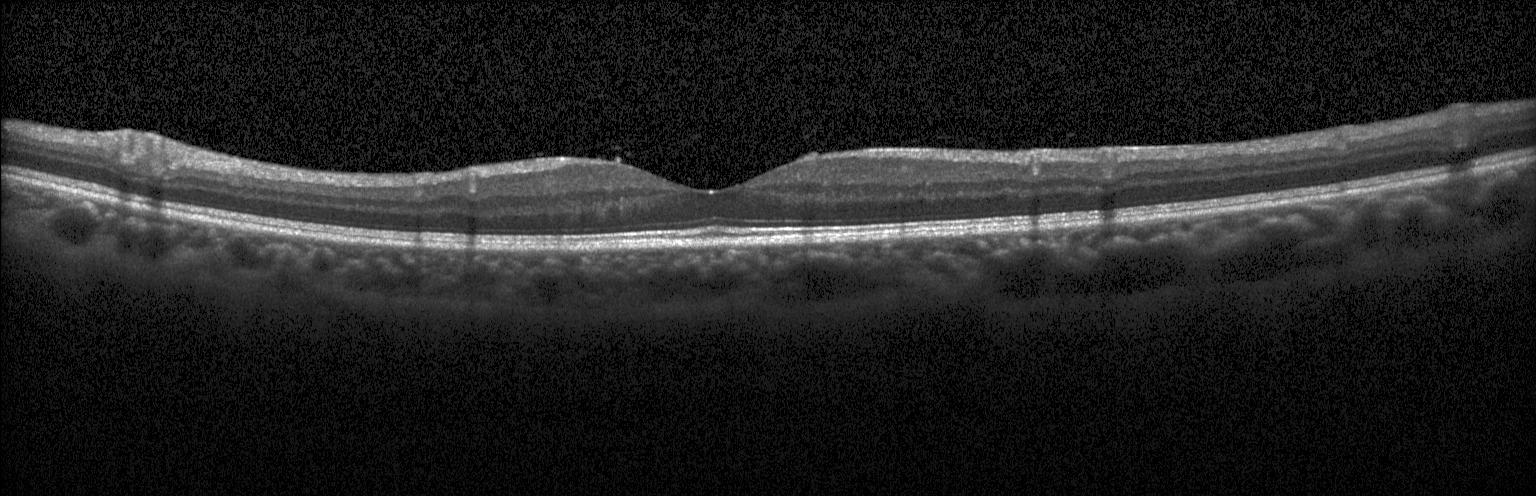
Diagnosis: no choroidal neovascularization, diabetic macular edema, or drusen.